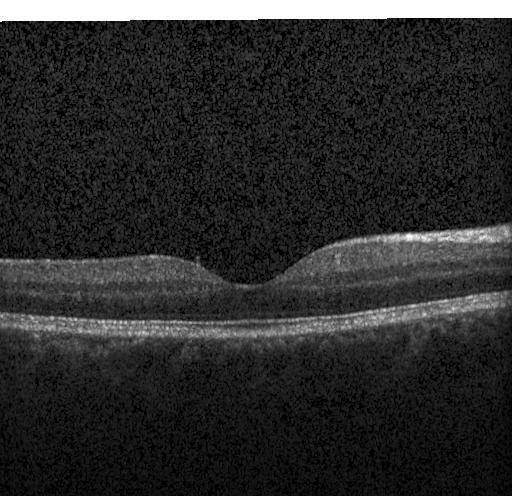 OCT B-scan.
Dx: no choroidal neovascularization, no diabetic macular edema, and no drusen.